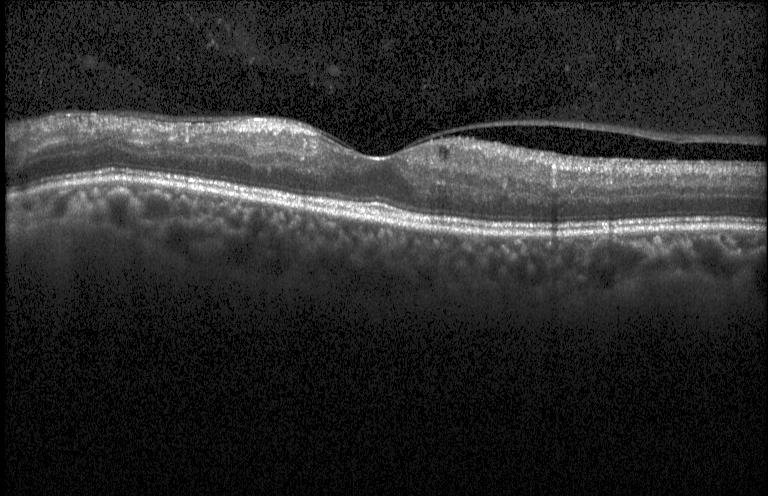

Dx: DME.